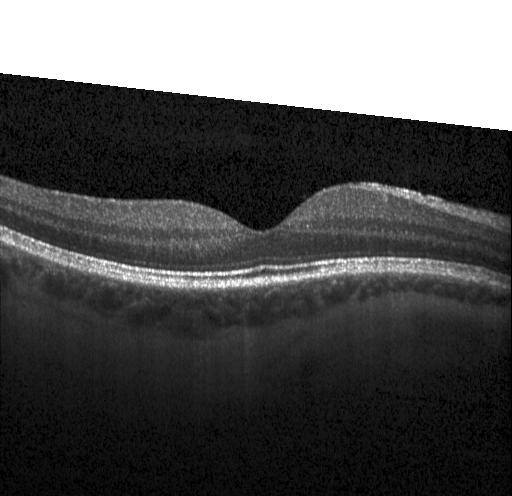
OCT B-scan; through the macula; SD-OCT. Neither CNV, DME, nor drusen.